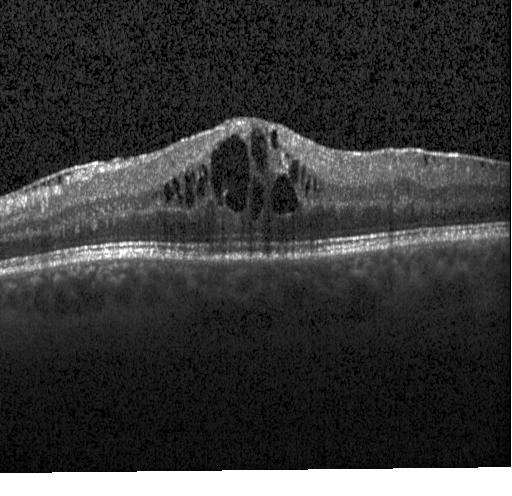 Through the macula · spectral-domain optical coherence tomography · retinal OCT cross-section.
The scan shows DME.